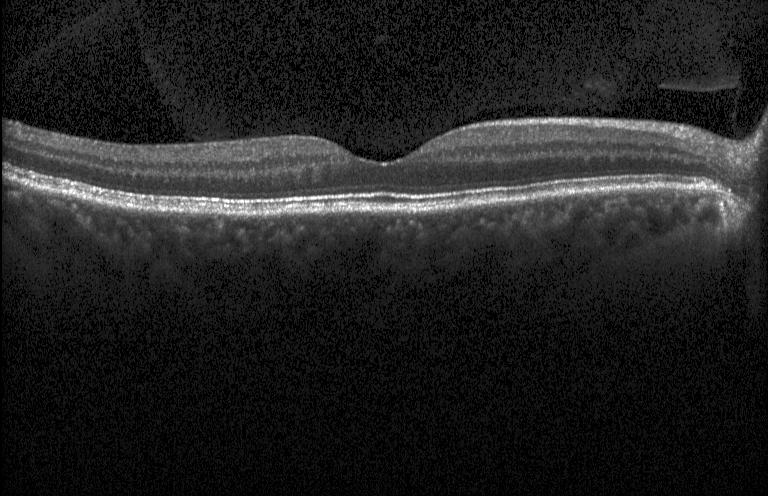 SD-OCT; optical coherence tomography B-scan — Impression: no CNV, no DME, and no drusen.